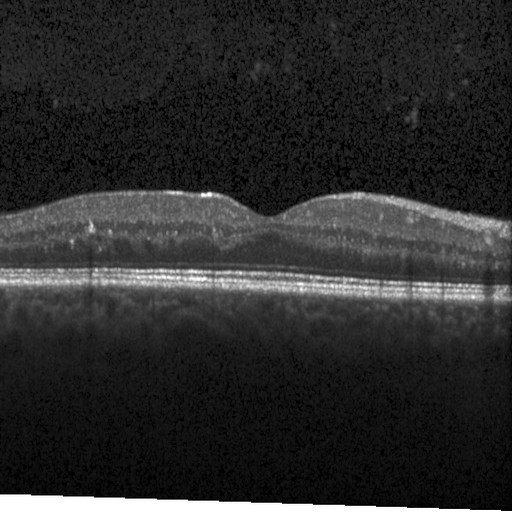
OCT line scan. Macular OCT: DME.